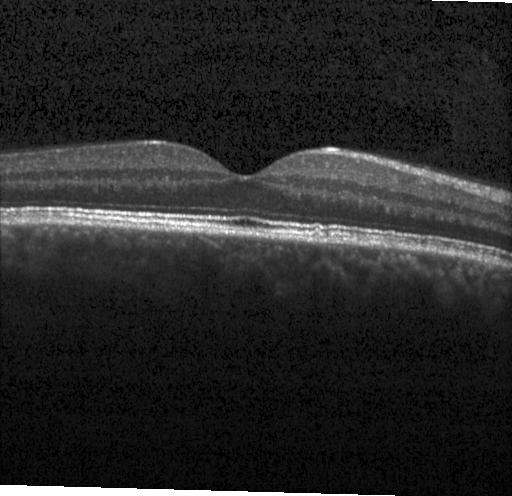

OCT line scan, horizontal scan through the fovea. Impression: no evidence of choroidal neovascularization, diabetic macular edema, or drusen.